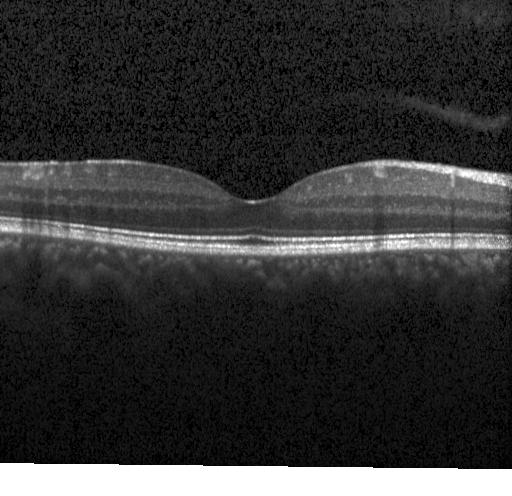
Centered on the fovea, spectral-domain OCT, optical coherence tomography B-scan, Heidelberg Spectralis.
Assessment: no choroidal neovascularization, diabetic macular edema, or drusen.